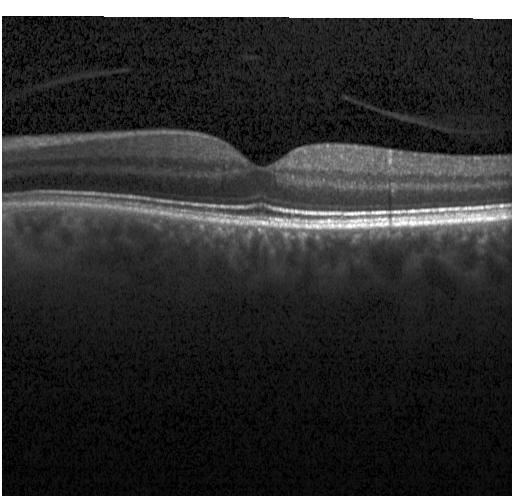
Optical coherence tomography scan.
Assessment: neither choroidal neovascularization, diabetic macular edema, nor drusen.